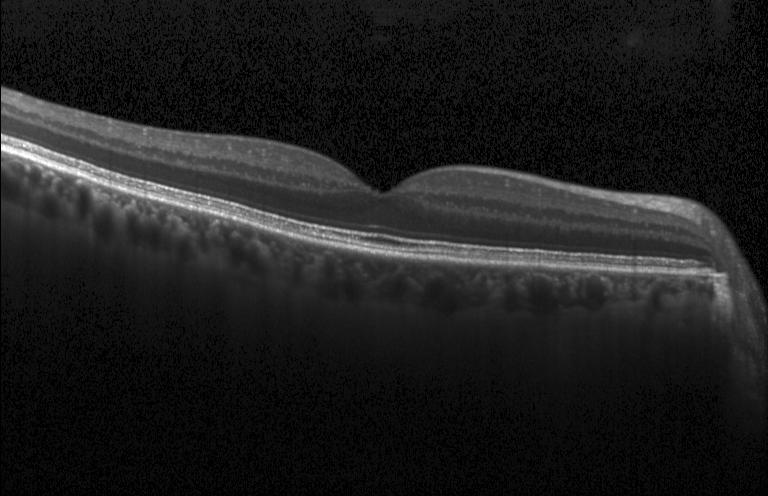
Optical coherence tomography scan
Neither CNV, DME, nor drusen.